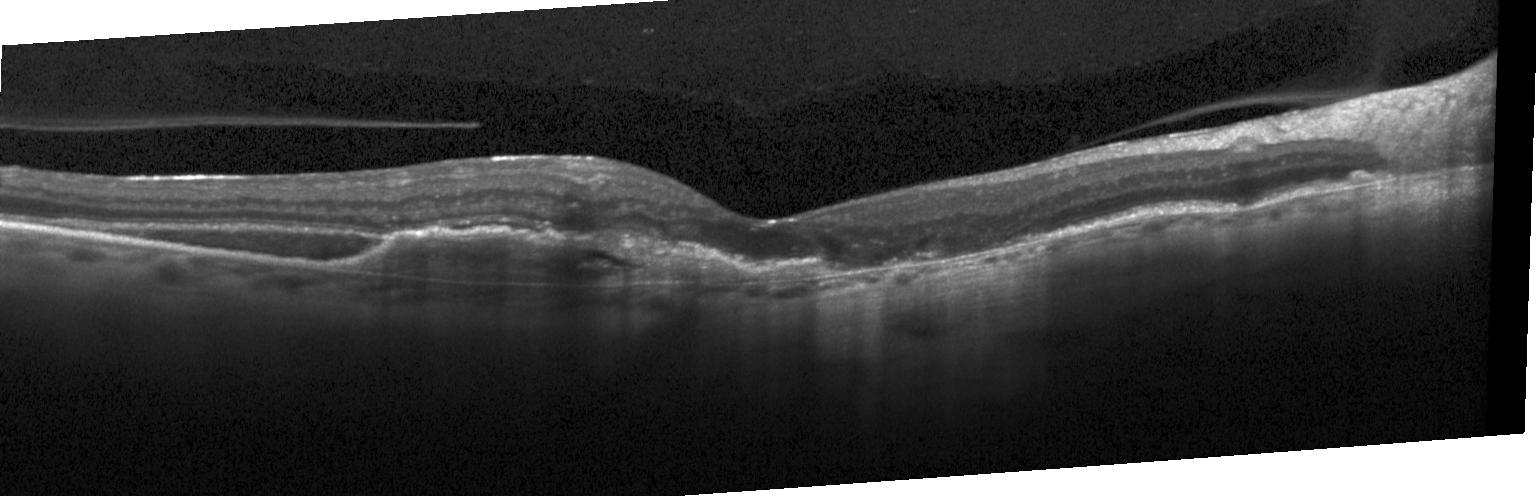 Spectral-domain optical coherence tomography, OCT B-scan, Heidelberg Spectralis OCT system — This B-scan demonstrates choroidal neovascularization.